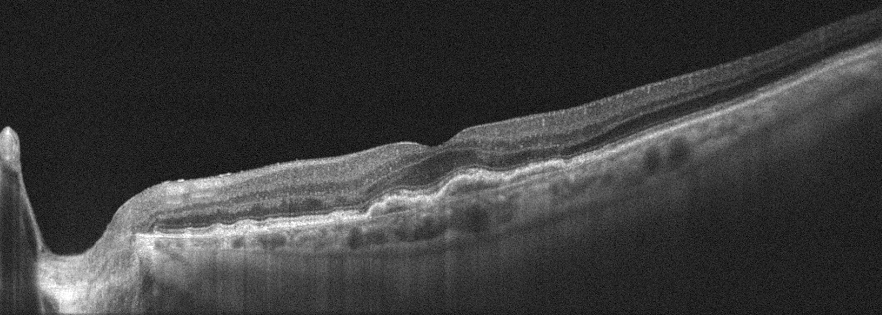

The scan shows AMD.